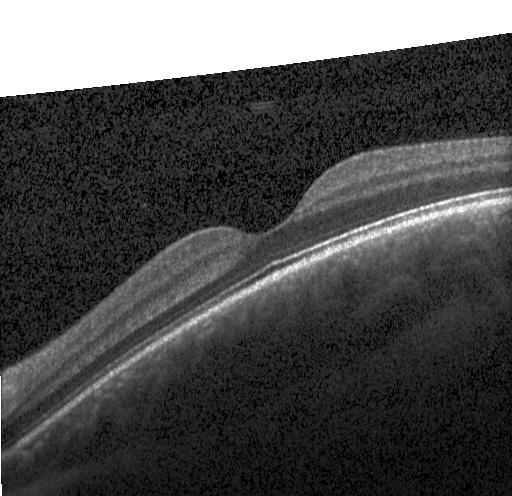

OCT B-scan. The scan shows no choroidal neovascularization, diabetic macular edema, or drusen.